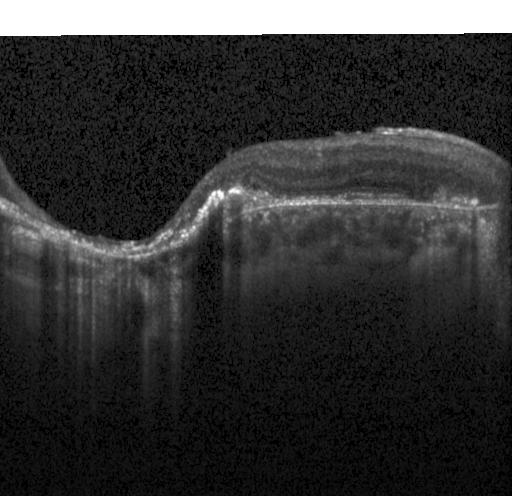

Impression: choroidal neovascularization.